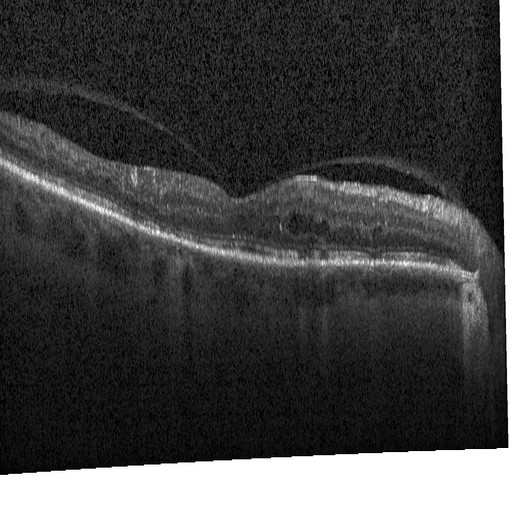

Instrument: Heidelberg Spectralis · optical coherence tomography B-scan
Macular OCT: diabetic macular edema (DME).